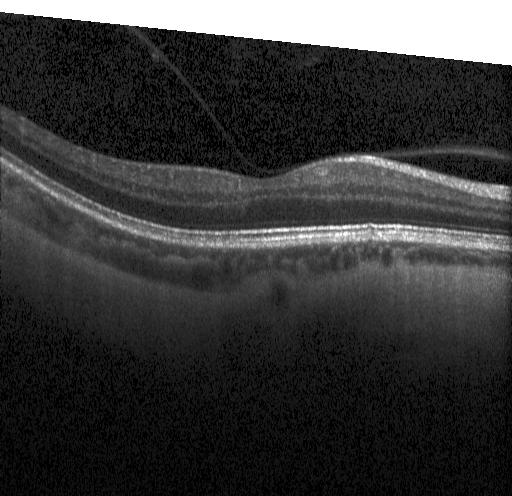
Instrument: Heidelberg Spectralis, OCT line scan, spectral-domain OCT
Diagnosis: neither choroidal neovascularization, diabetic macular edema, nor drusen.